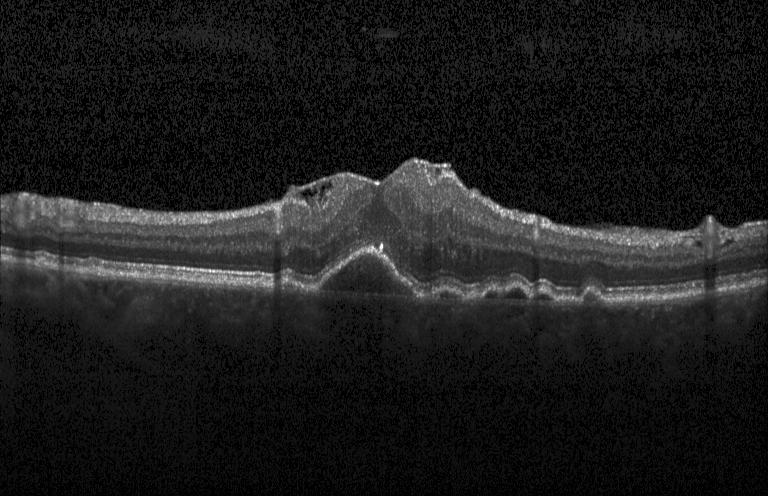 Retinal OCT B-scan. OCT finding: CNV.